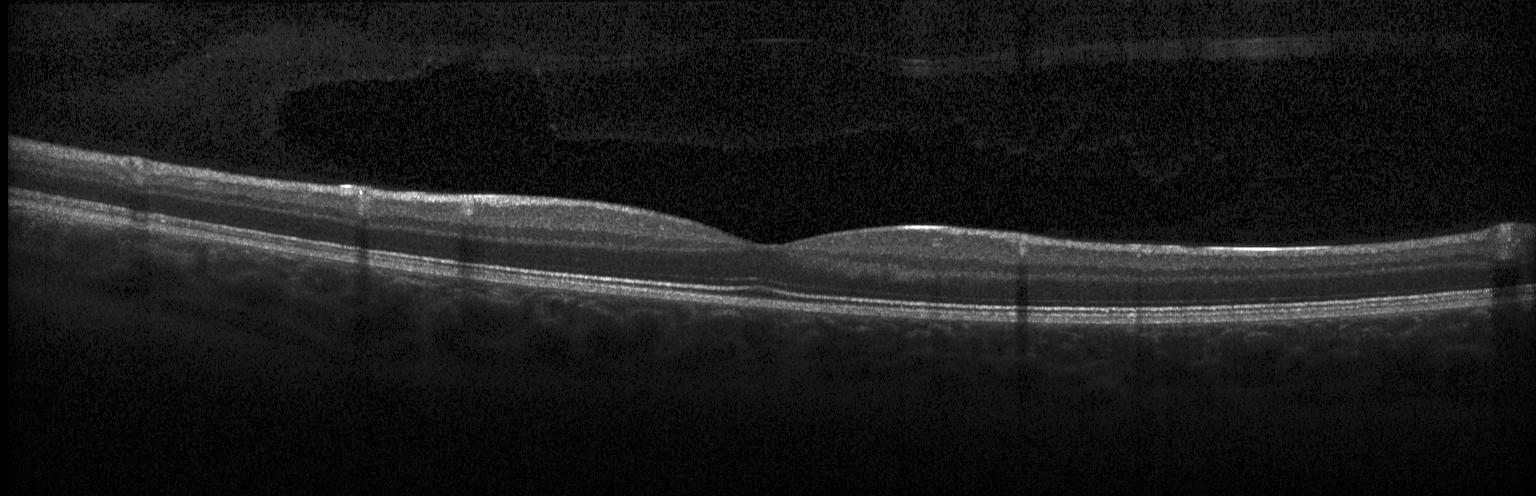 Macular OCT: no evidence of choroidal neovascularization, diabetic macular edema, or drusen.